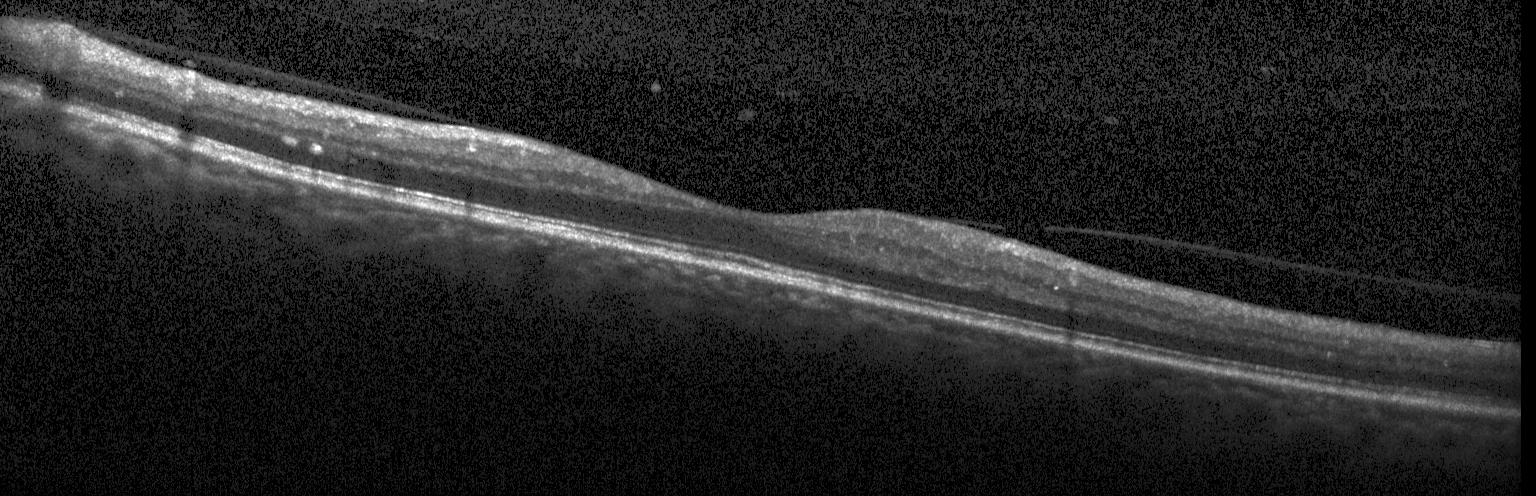

SD-OCT. Optical coherence tomography scan. Through the macula. Instrument: Heidelberg Spectralis
The scan shows no choroidal neovascularization, no diabetic macular edema, and no drusen.